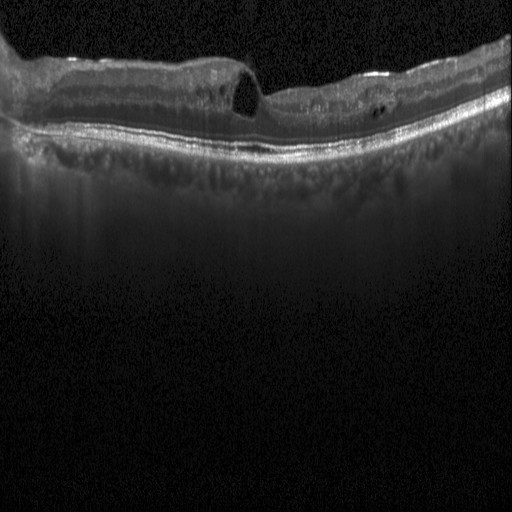 Heidelberg Spectralis · macular scan · optical coherence tomography B-scan — This B-scan demonstrates DME.